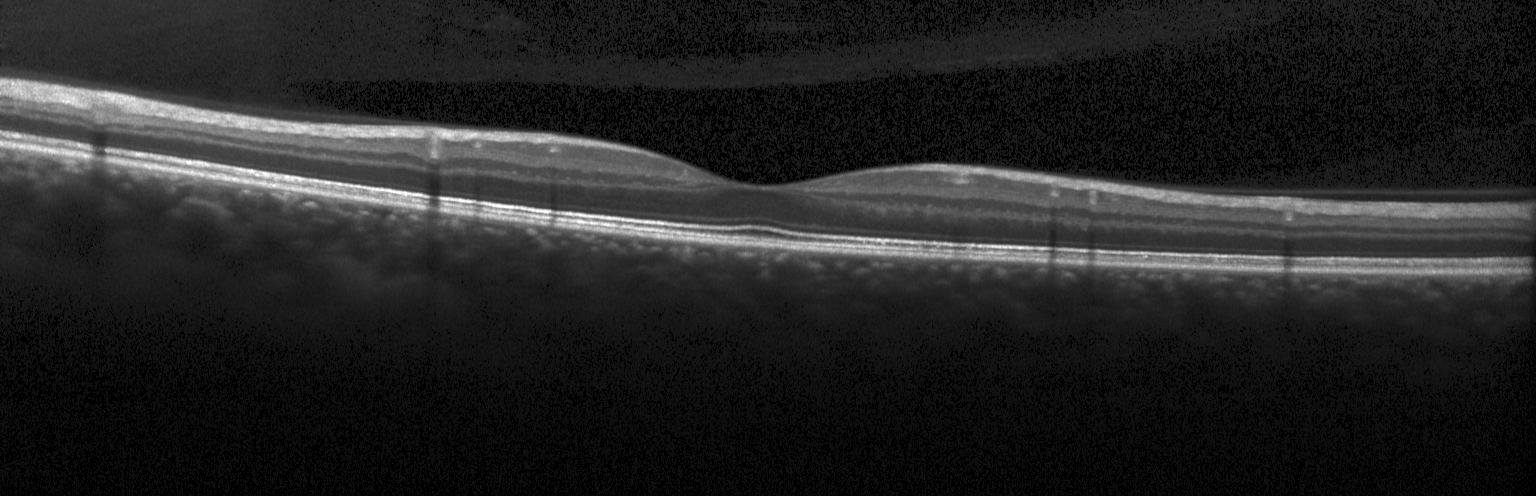 Centered on the fovea · instrument: Heidelberg Spectralis · spectral-domain optical coherence tomography · retinal OCT B-scan.
Diagnosis: no CNV, DME, or drusen.